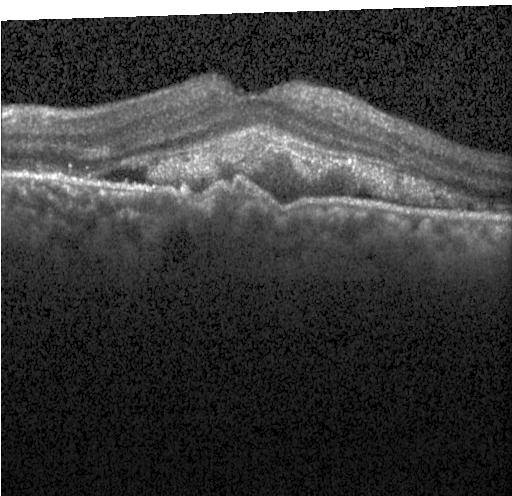

Optical coherence tomography B-scan. Instrument: Heidelberg Spectralis. Spectral-domain OCT.
Assessment: choroidal neovascularization.